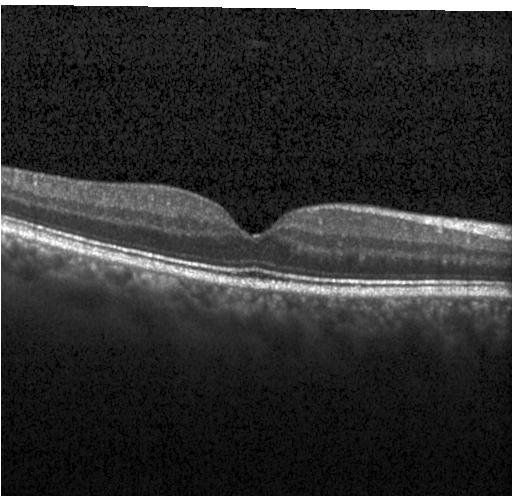

SD-OCT · retinal OCT cross-section. Finding: neither choroidal neovascularization, diabetic macular edema, nor drusen.